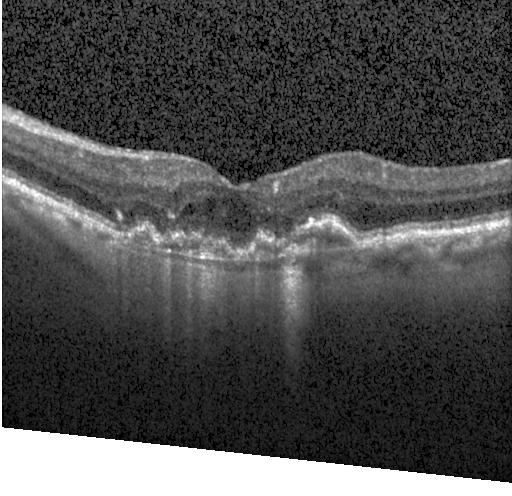

Spectral-domain optical coherence tomography · acquired on a Heidelberg Spectralis · OCT B-scan — Dx: a choroidal neovascular membrane.